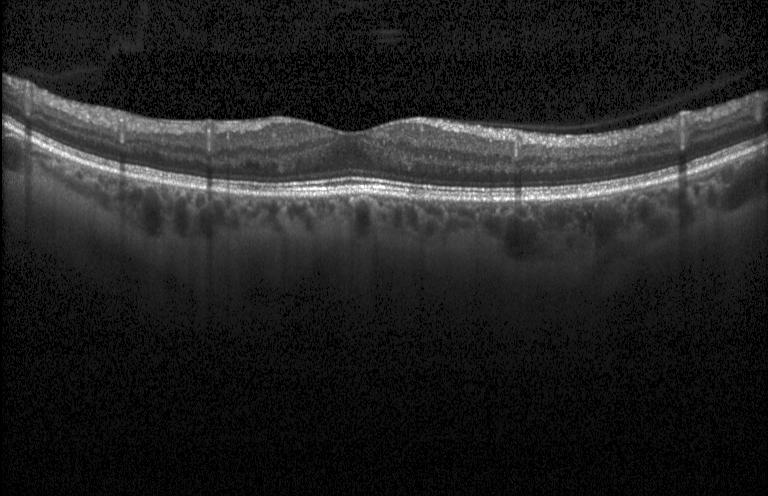
Optical coherence tomography B-scan · through the macula · SD-OCT · acquired on a Heidelberg Spectralis. Diagnosis: neither choroidal neovascularization, diabetic macular edema, nor drusen.